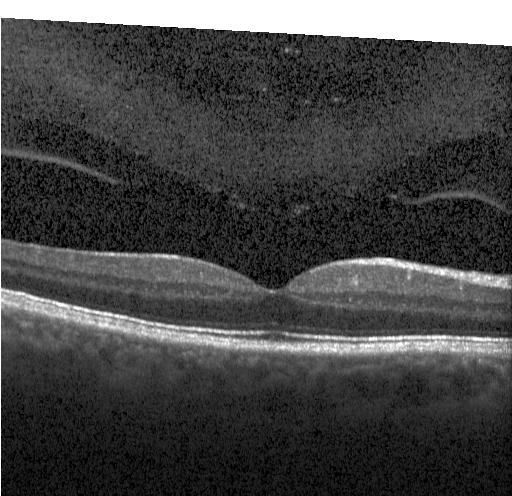 OCT B-scan, macular scan, Heidelberg Spectralis — Macular OCT: no CNV, no DME, and no drusen.